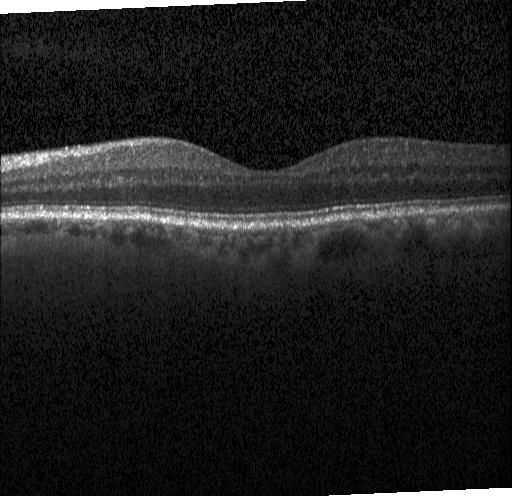
Retinal OCT cross-section.
Assessment: neither choroidal neovascularization, diabetic macular edema, nor drusen.